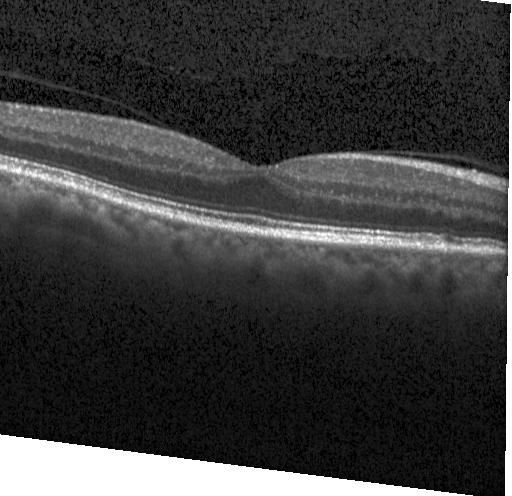
Impression: no choroidal neovascularization, no diabetic macular edema, and no drusen.